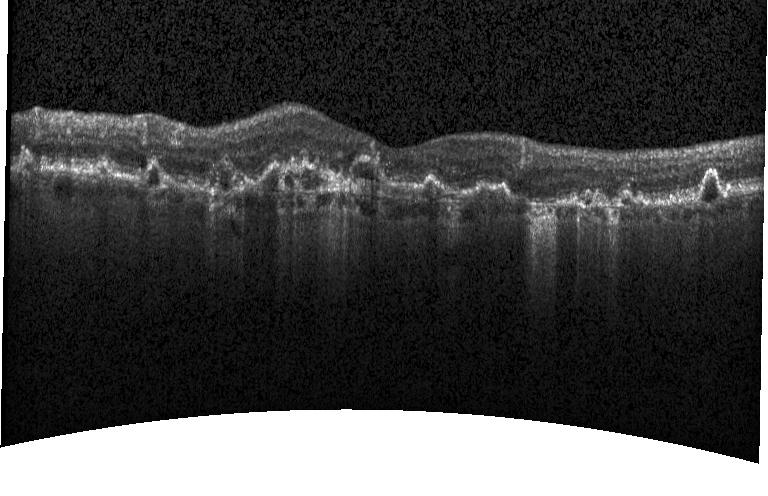

Macular scan, optical coherence tomography scan, spectral-domain OCT.
A choroidal neovascular membrane.